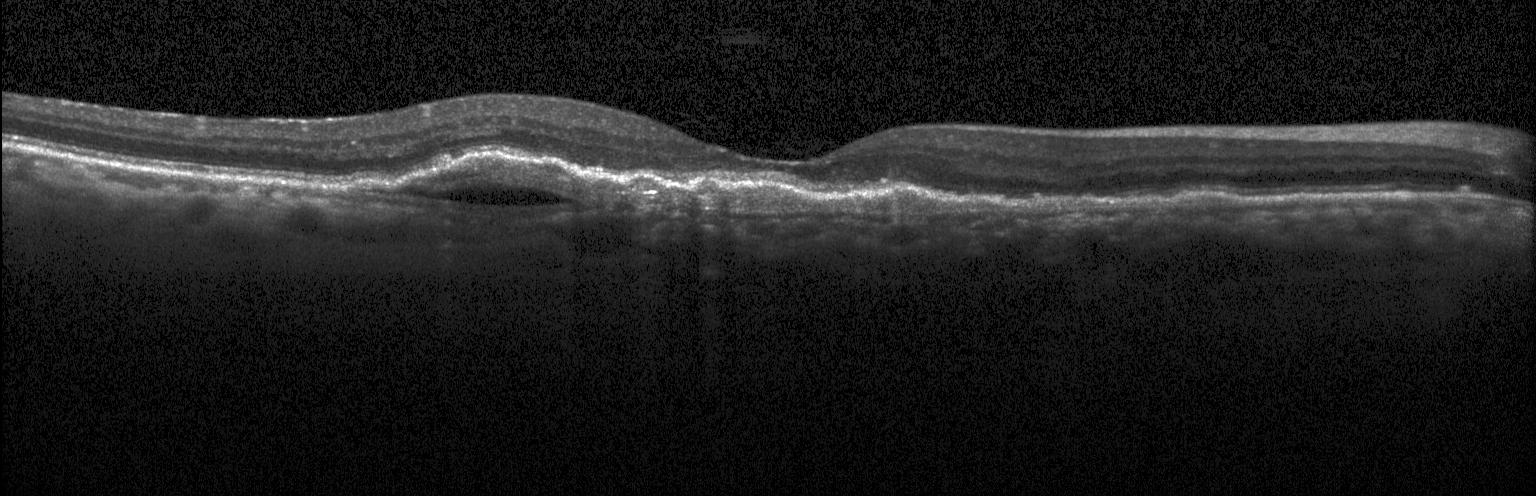

Optical coherence tomography B-scan; acquired on a Heidelberg Spectralis; fovea-centered. Macular OCT: a choroidal neovascular membrane.